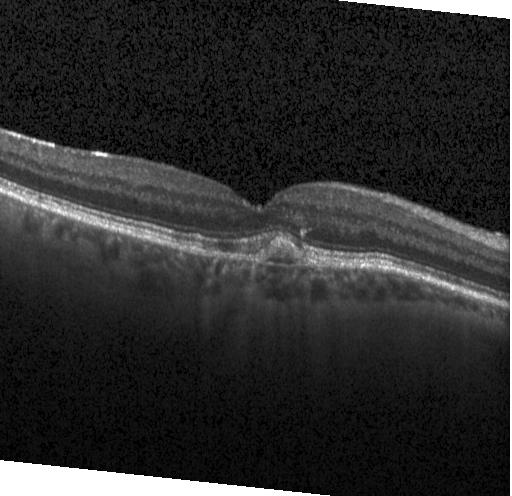

OCT finding: CNV.